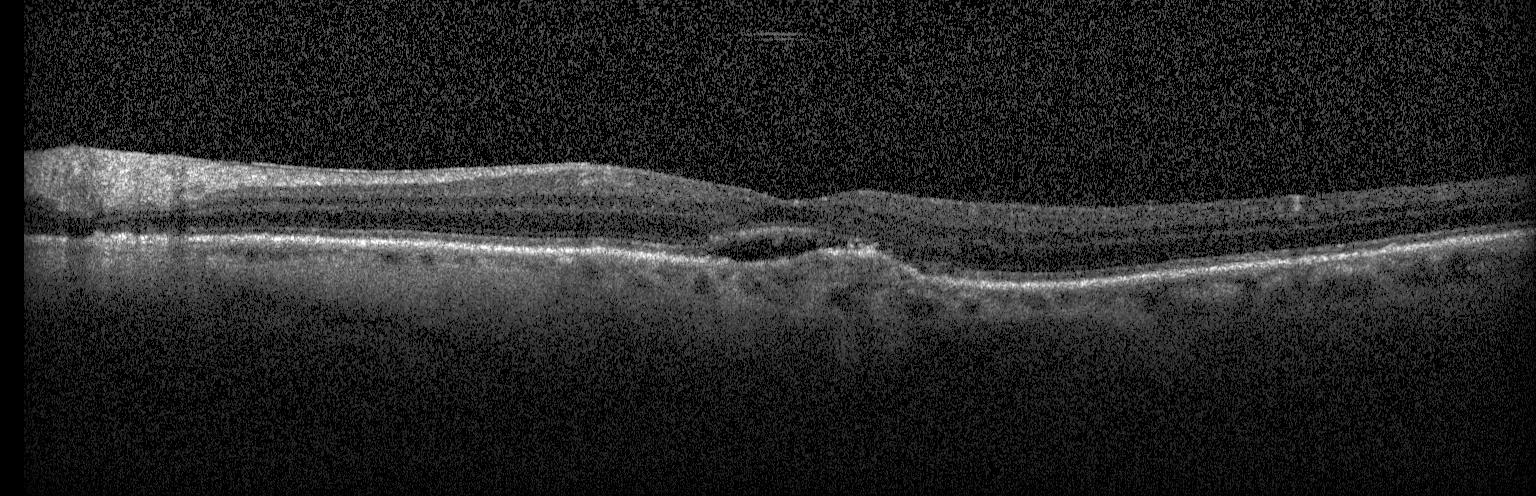 Heidelberg Spectralis. Fovea-centered. OCT line scan. OCT finding: choroidal neovascularization (CNV).